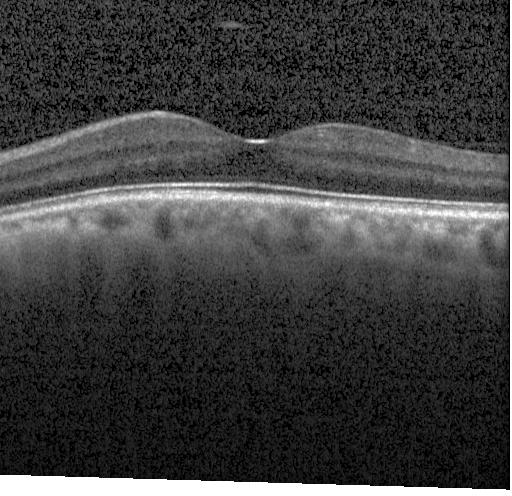 Macular OCT demonstrating no evidence of choroidal neovascularization, diabetic macular edema, or drusen.